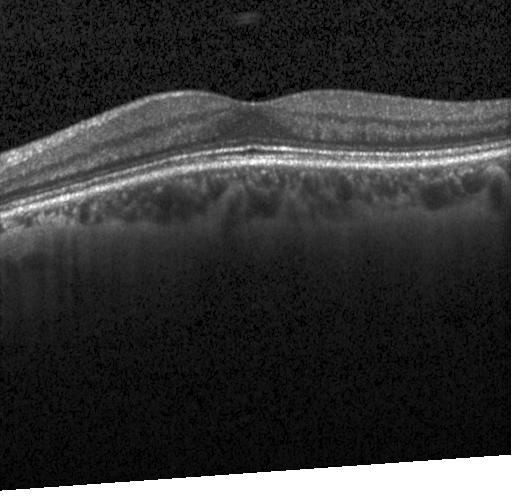

Acquired on a Heidelberg Spectralis; retinal OCT B-scan; fovea-centered
Impression: no choroidal neovascularization, no diabetic macular edema, and no drusen.